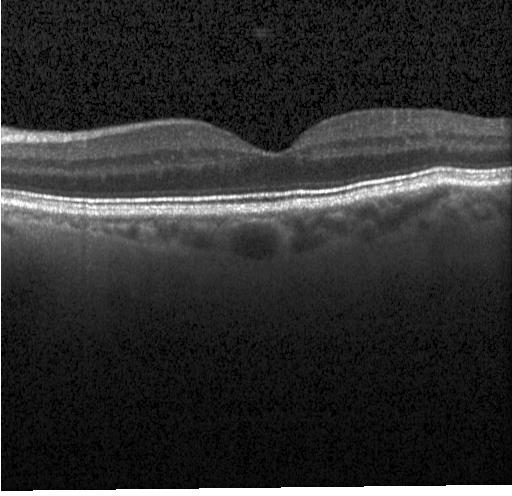

Impression: no evidence of choroidal neovascularization, diabetic macular edema, or drusen.